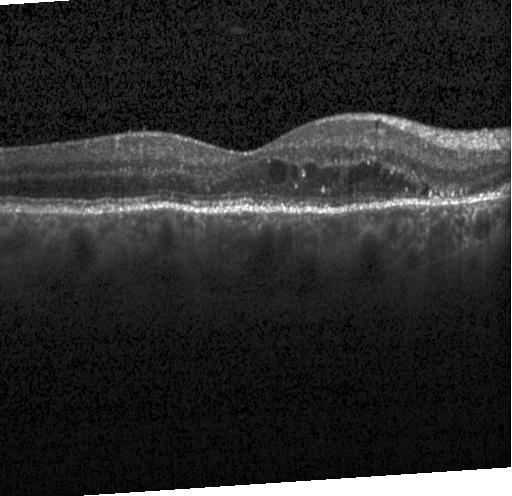
Impression: diabetic macular edema (DME).